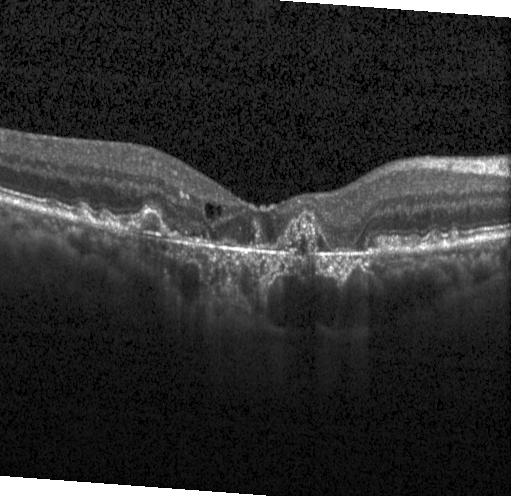 OCT line scan.
Impression: CNV.